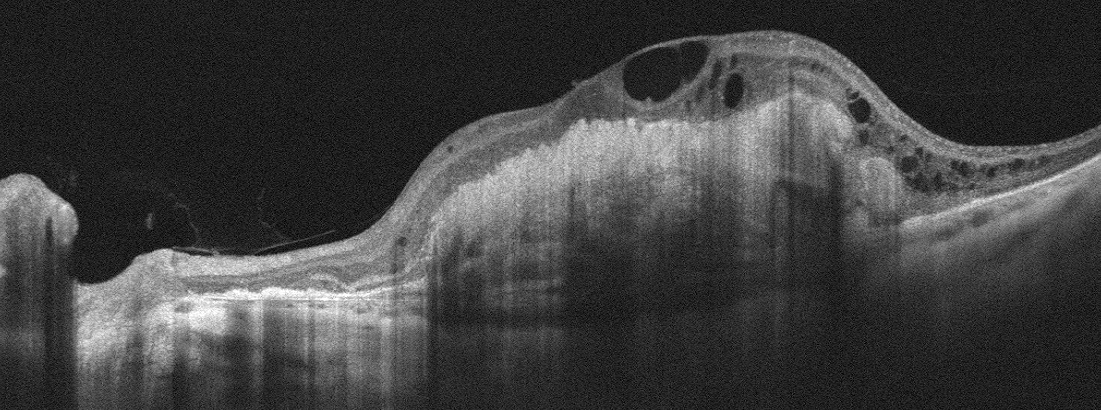
Dx: AMD.